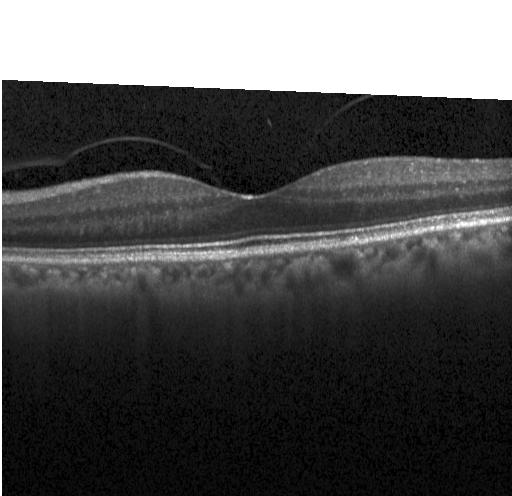 Finding: no evidence of choroidal neovascularization, diabetic macular edema, or drusen.